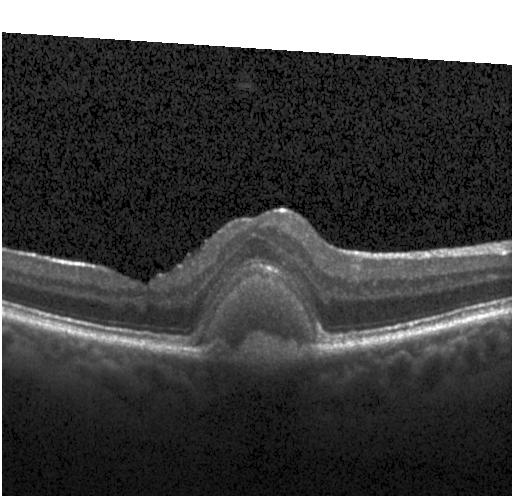
Spectral-domain optical coherence tomography; macular scan; Heidelberg Spectralis; retinal OCT cross-section
Dx: choroidal neovascularization (CNV).